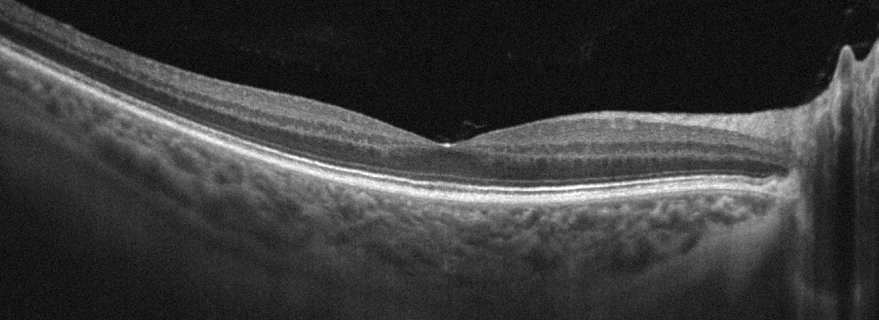
Finding: no AMD, DME, ERM, RAO, RVO, or VID.